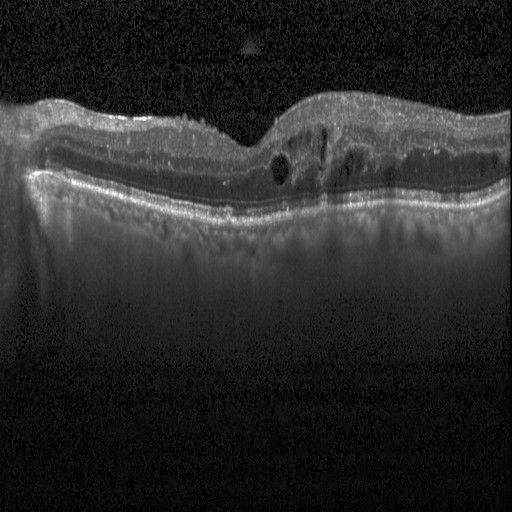
Impression: diabetic macular edema (DME).